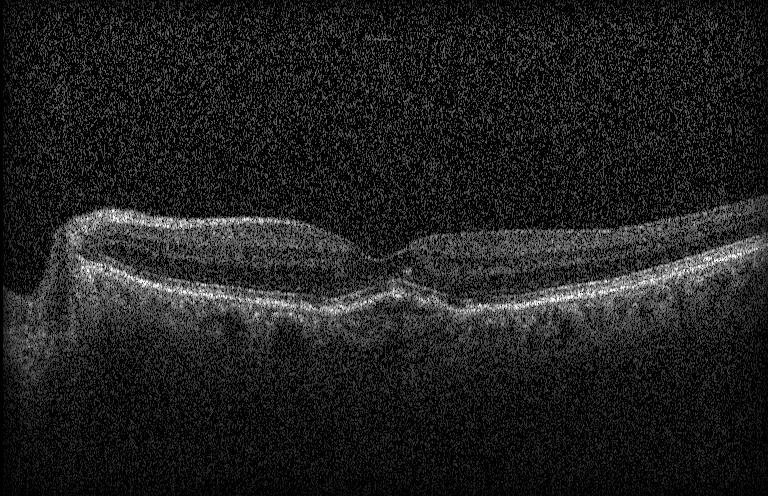 Retinal OCT cross-section.
Impression: a choroidal neovascular membrane.